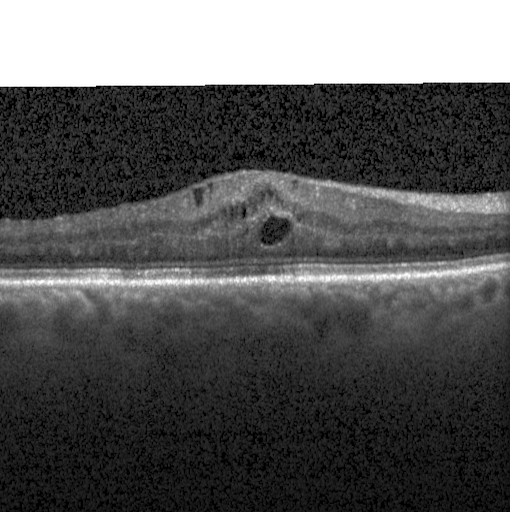

Retinal OCT cross-section, SD-OCT, centered on the fovea.
Impression: DME.